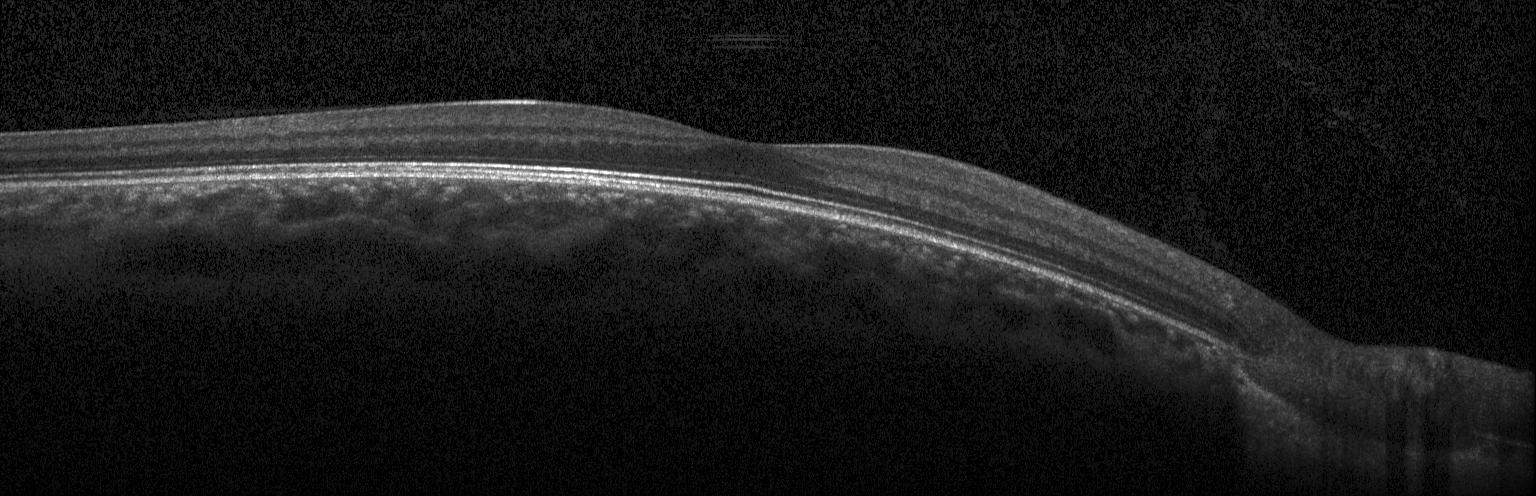
OCT B-scan · centered on the fovea · spectral-domain optical coherence tomography · instrument: Heidelberg Spectralis.
Finding: neither CNV, DME, nor drusen.